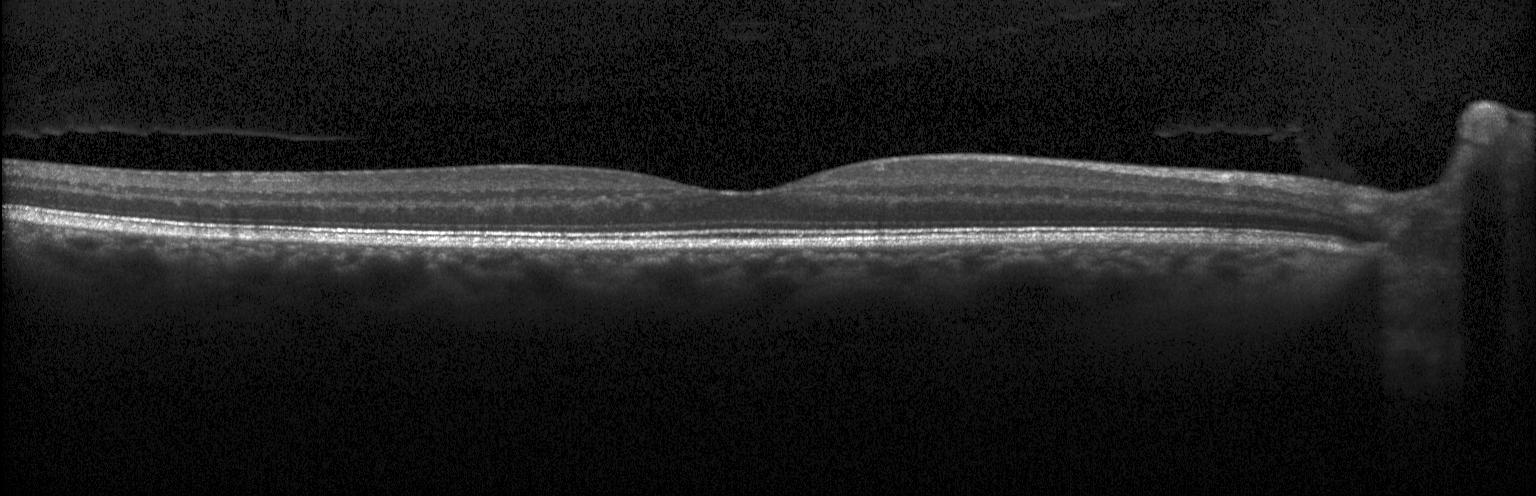 Retinal OCT B-scan. Impression: no choroidal neovascularization, no diabetic macular edema, and no drusen.